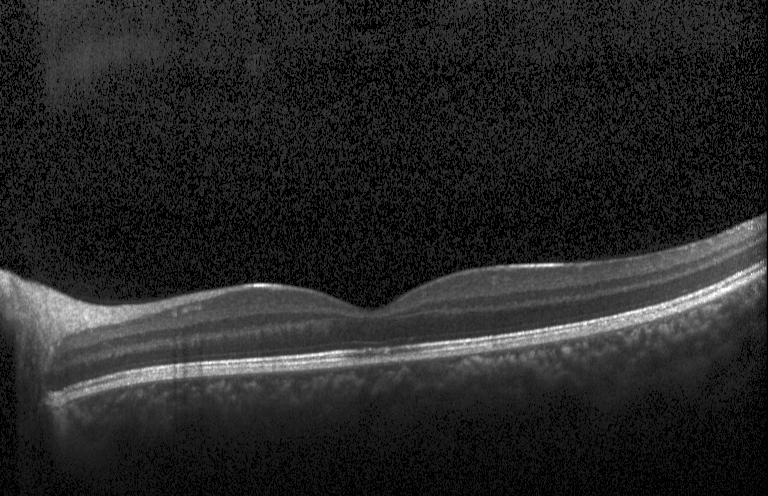

OCT B-scan.
OCT finding: no CNV, DME, or drusen.